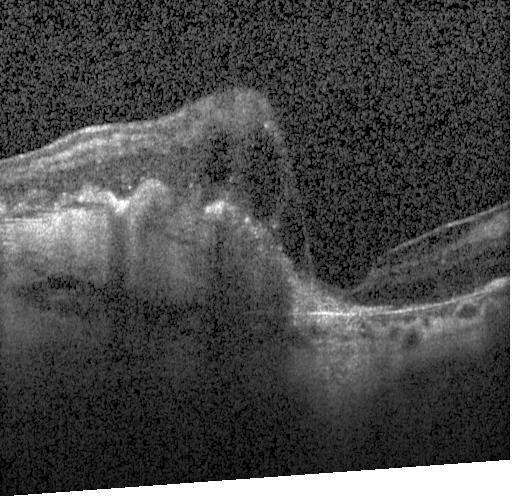
Optical coherence tomography scan · SD-OCT · fovea-centered · Heidelberg Spectralis
Diagnosis: choroidal neovascularization (CNV).